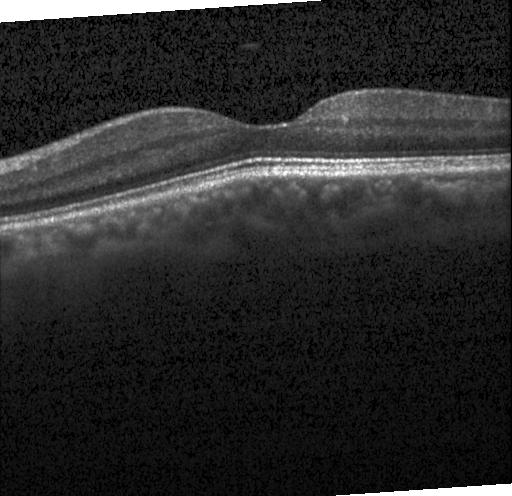 Optical coherence tomography B-scan. Macular scan. SD-OCT — Finding: no evidence of choroidal neovascularization, diabetic macular edema, or drusen.